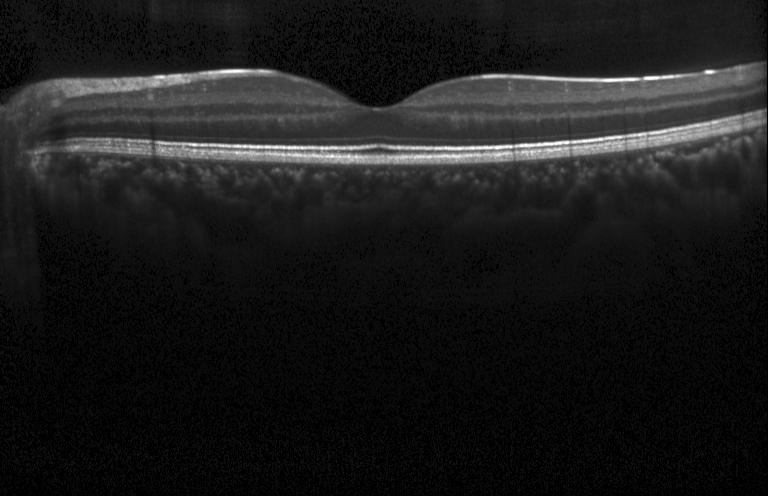
The scan shows no choroidal neovascularization, no diabetic macular edema, and no drusen.